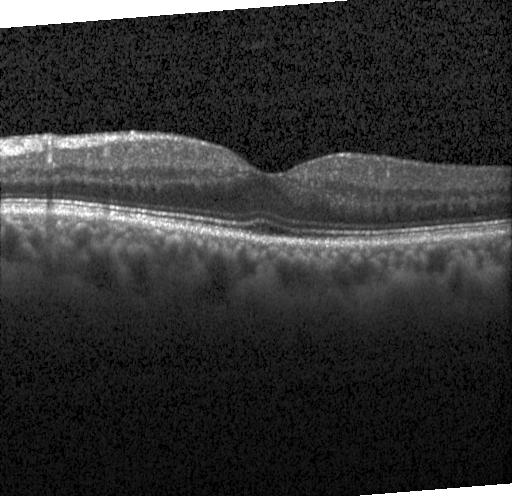

Spectral-domain OCT · retinal OCT cross-section — Impression: no evidence of CNV, DME, or drusen.